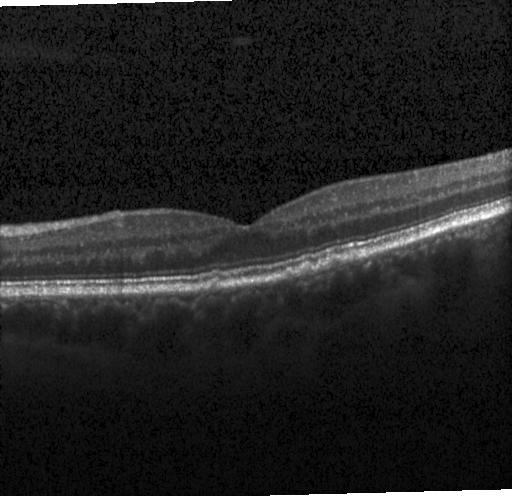
Diagnosis: sub-RPE drusenoid deposits.